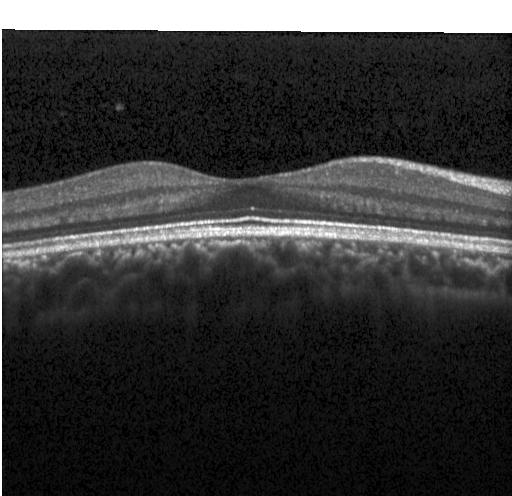 Optical coherence tomography scan · Heidelberg Spectralis OCT system · horizontal scan through the fovea. Diagnosis: no choroidal neovascularization, diabetic macular edema, or drusen.